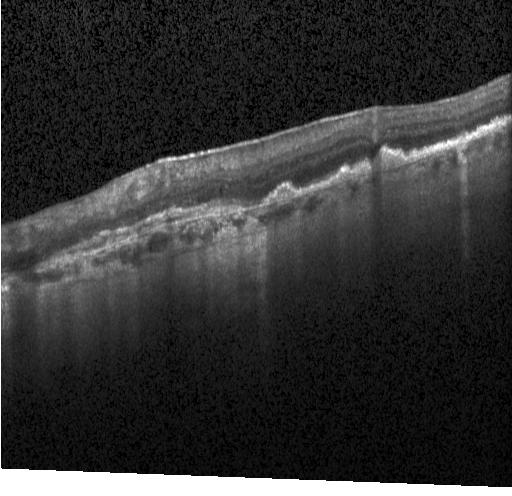

Spectral-domain OCT; Heidelberg Spectralis OCT system; retinal OCT cross-section; macular scan.
This B-scan demonstrates choroidal neovascularization.